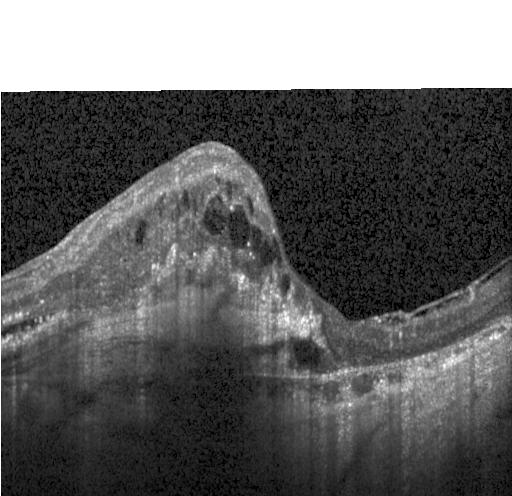
Diagnosis: a choroidal neovascular membrane.